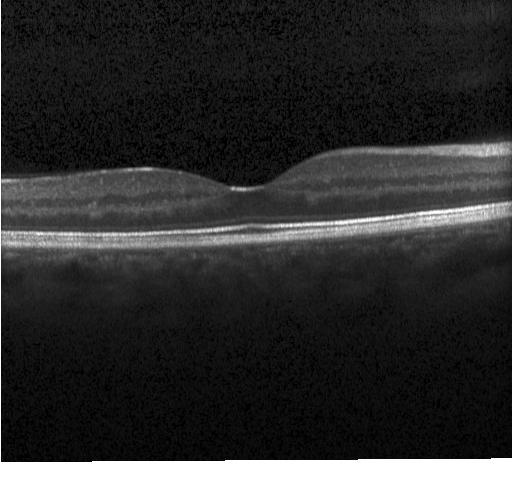 Diagnosis: no evidence of choroidal neovascularization, diabetic macular edema, or drusen.